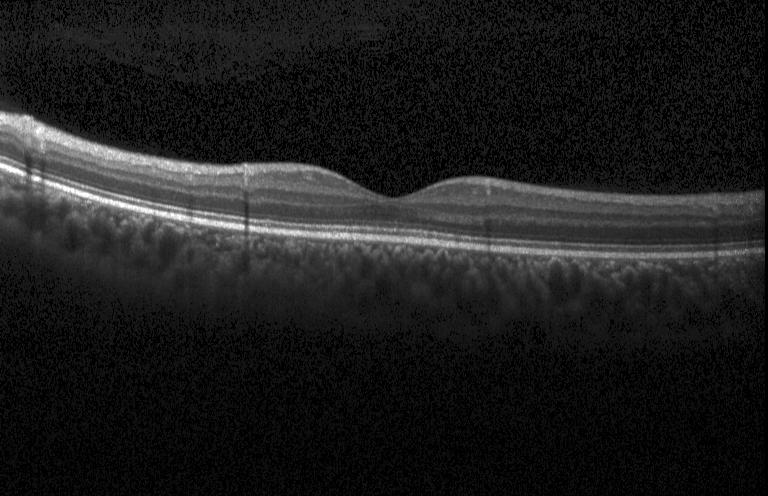
Spectral-domain optical coherence tomography · through the macula · instrument: Heidelberg Spectralis · OCT line scan — Impression: no evidence of CNV, DME, or drusen.